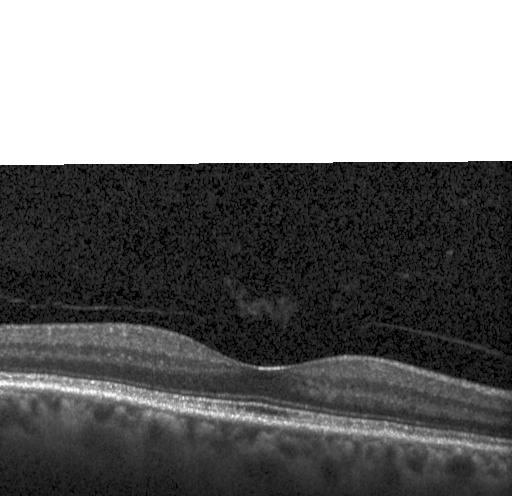

OCT finding: no CNV, no DME, and no drusen.